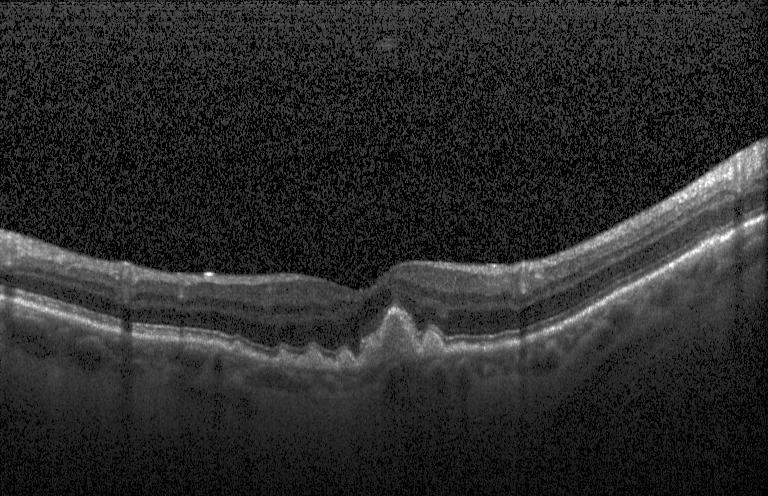

Retinal OCT cross-section showing sub-RPE drusenoid deposits.